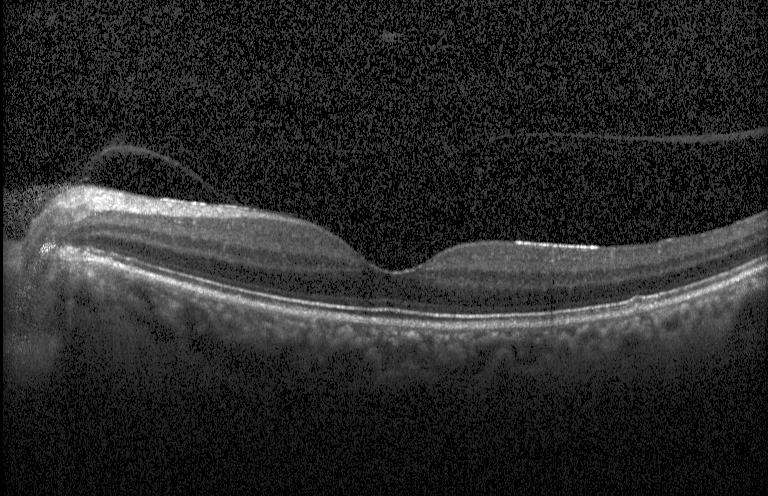

Macular OCT demonstrating neither choroidal neovascularization, diabetic macular edema, nor drusen.